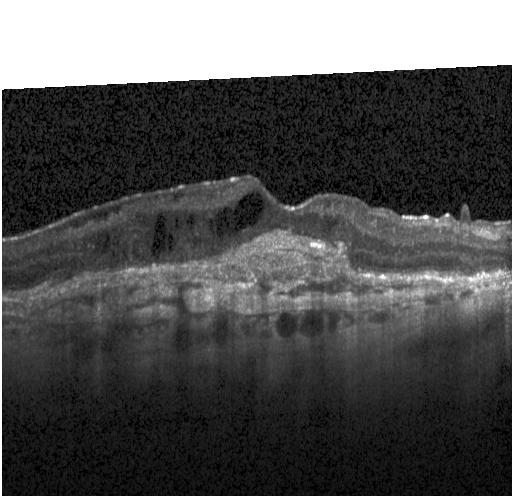 Acquired on a Heidelberg Spectralis · macular scan · spectral-domain OCT · retinal OCT cross-section.
OCT finding: choroidal neovascularization.